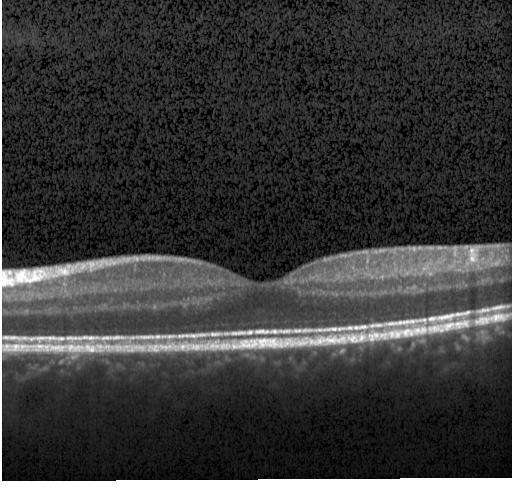 Retinal OCT cross-section showing no evidence of choroidal neovascularization, diabetic macular edema, or drusen.